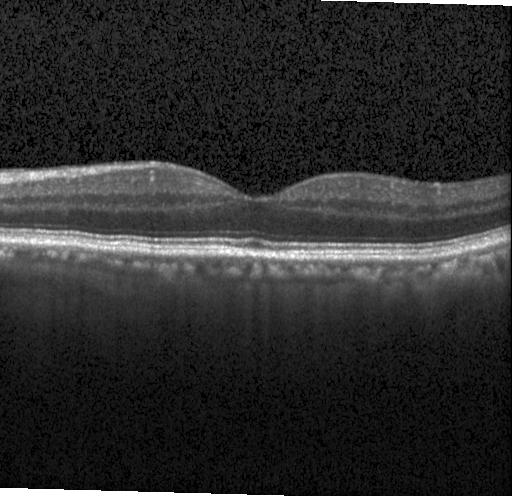

OCT line scan. Fovea-centered
Impression: no choroidal neovascularization, diabetic macular edema, or drusen.